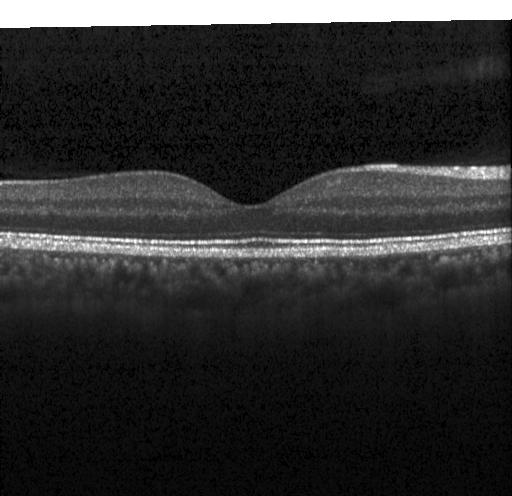

Impression: no evidence of CNV, DME, or drusen.